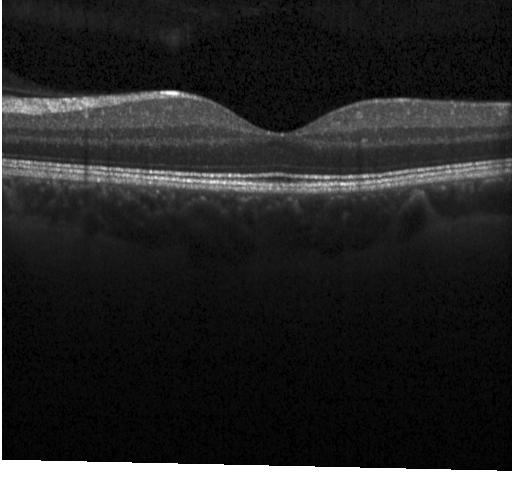

Assessment: no choroidal neovascularization, diabetic macular edema, or drusen.